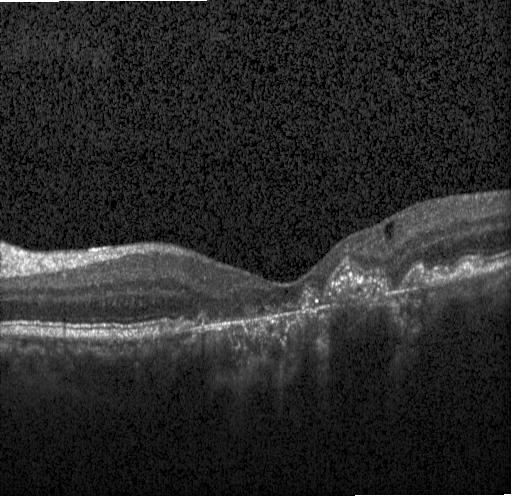 Macular OCT demonstrating choroidal neovascularization.